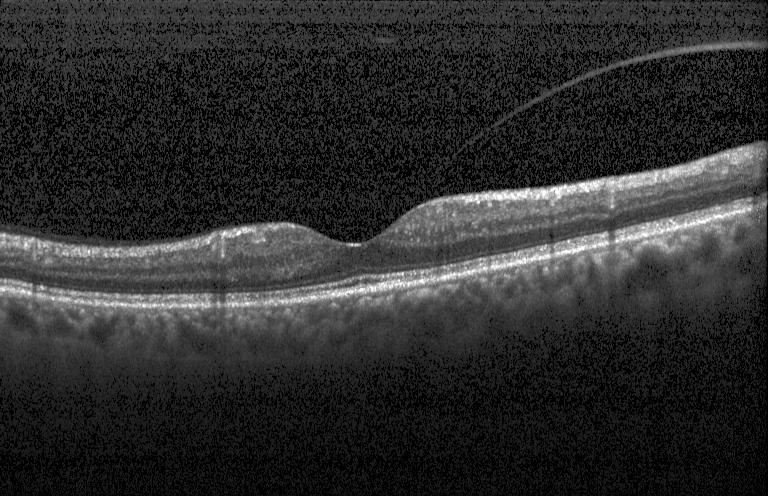

OCT line scan · macular scan.
Assessment: no choroidal neovascularization, diabetic macular edema, or drusen.